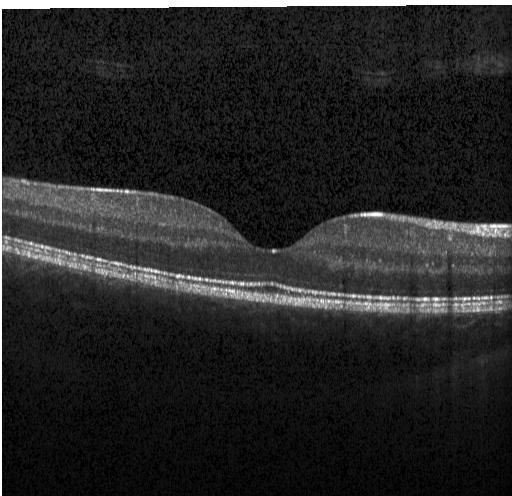

Optical coherence tomography B-scan — Dx: no choroidal neovascularization, diabetic macular edema, or drusen.